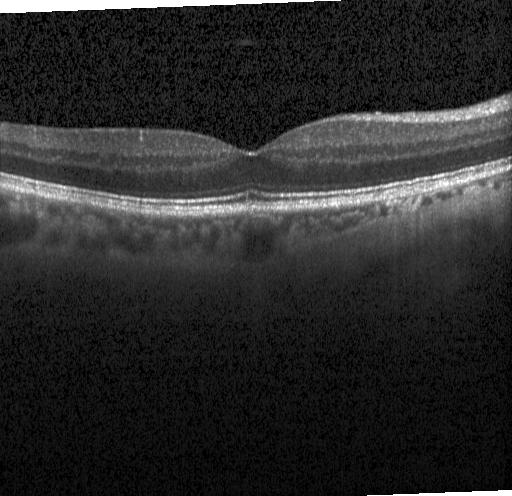
Retinal OCT cross-section.
Diagnosis: no evidence of CNV, DME, or drusen.